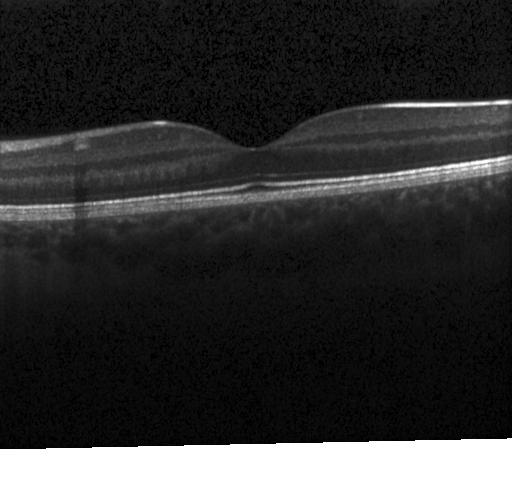
Spectral-domain OCT; optical coherence tomography scan; fovea-centered; acquired on a Heidelberg Spectralis
Diagnosis: no choroidal neovascularization, no diabetic macular edema, and no drusen.